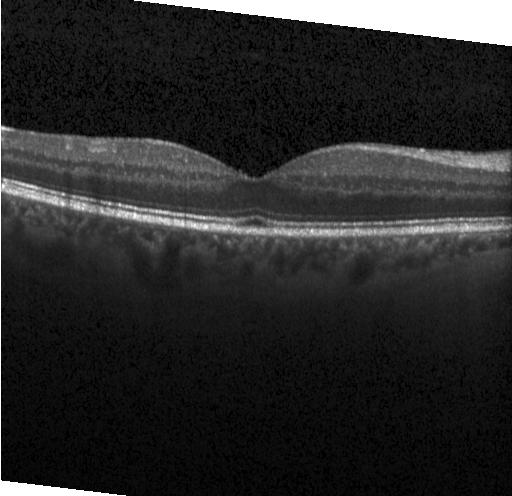
OCT line scan. Spectral-domain optical coherence tomography. Horizontal scan through the fovea. Heidelberg Spectralis OCT system. This B-scan demonstrates no choroidal neovascularization, diabetic macular edema, or drusen.